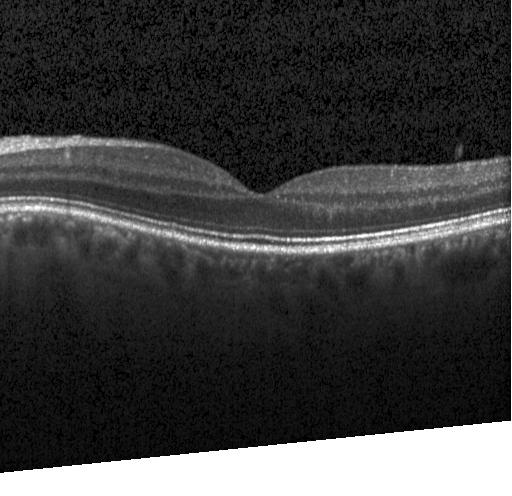
Retinal OCT B-scan. Finding: no evidence of choroidal neovascularization, diabetic macular edema, or drusen.